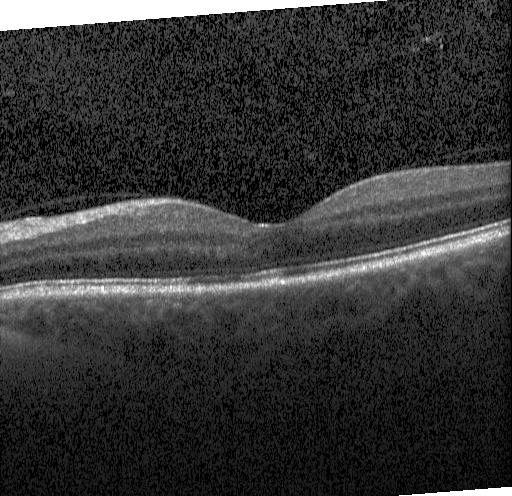 Centered on the fovea; retinal OCT B-scan. Macular OCT: no evidence of CNV, DME, or drusen.